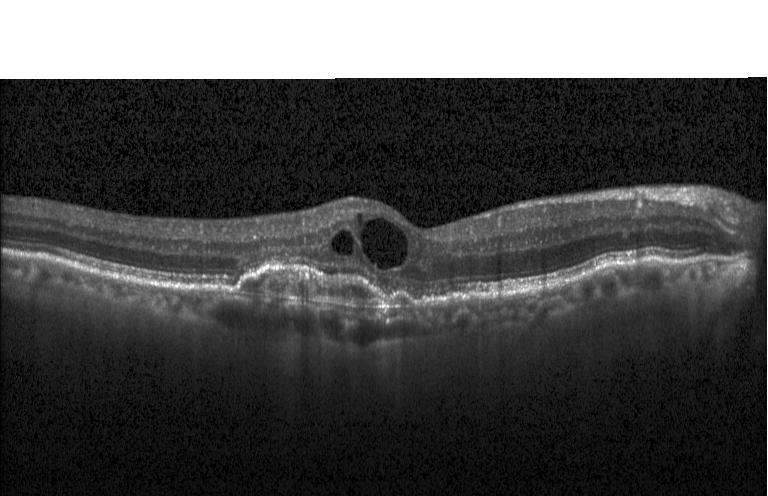 Optical coherence tomography scan.
Finding: CNV.